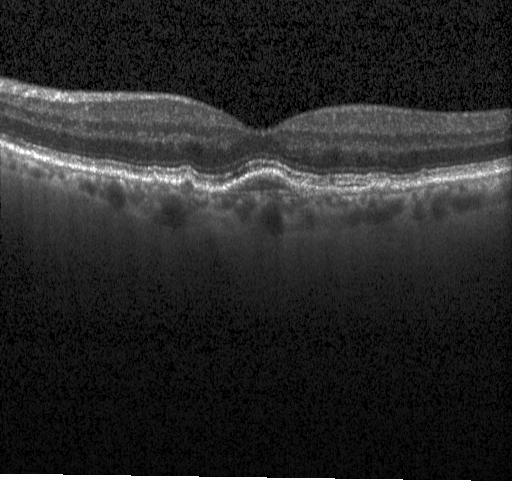
Assessment: a choroidal neovascular membrane.